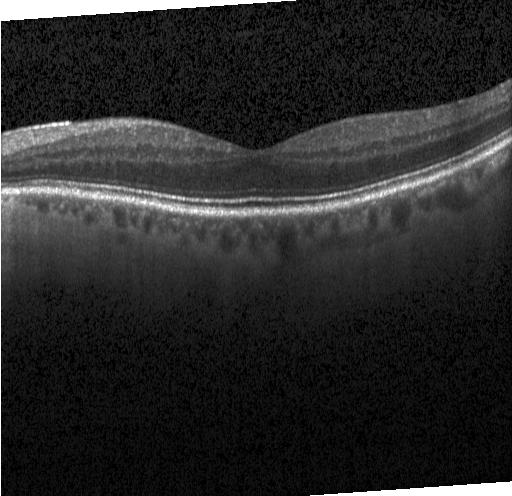 This B-scan demonstrates no CNV, no DME, and no drusen.